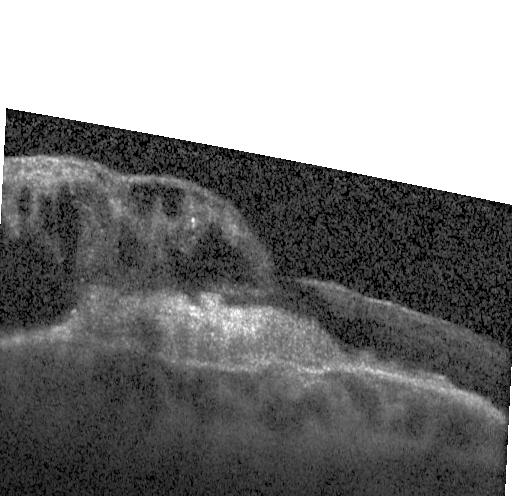

Heidelberg Spectralis; spectral-domain optical coherence tomography; fovea-centered; optical coherence tomography scan. Impression: a choroidal neovascular membrane.